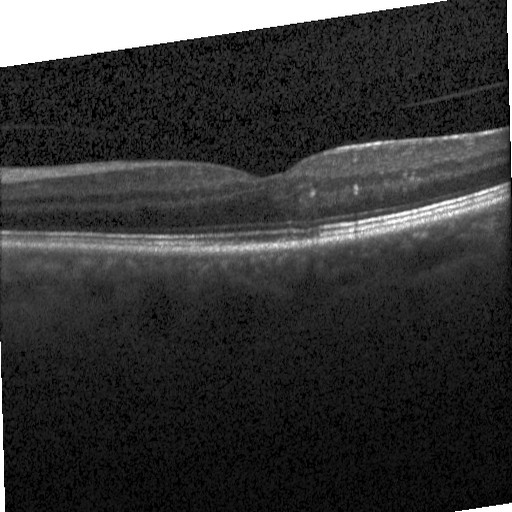
OCT finding: DME.